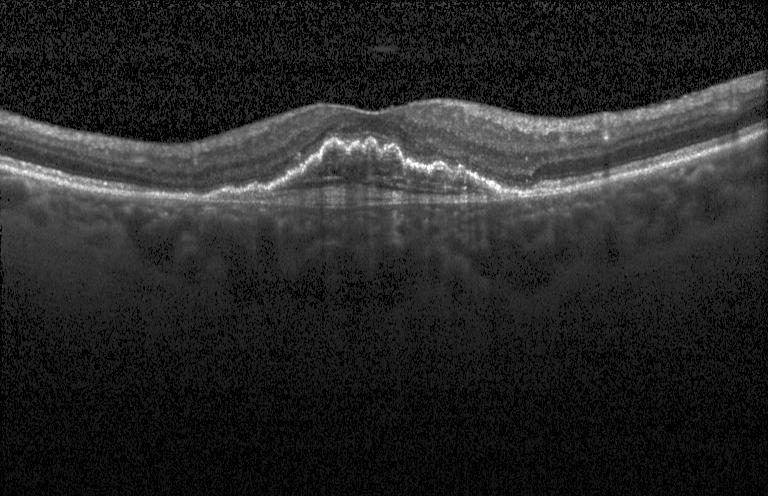
OCT B-scan. Macular OCT: a choroidal neovascular membrane.